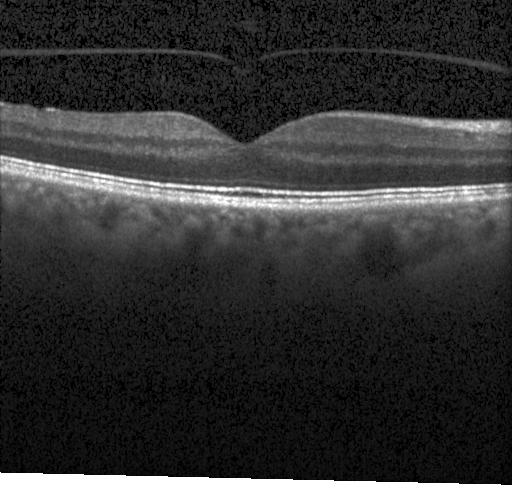

Assessment: no choroidal neovascularization, no diabetic macular edema, and no drusen.